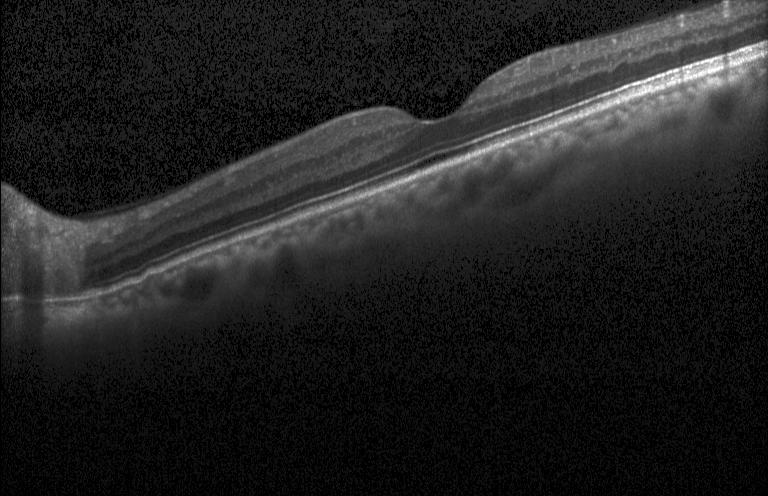

Retinal OCT B-scan
No evidence of choroidal neovascularization, diabetic macular edema, or drusen.